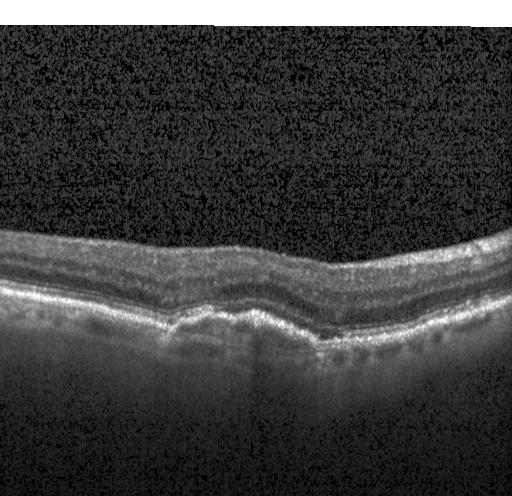
Impression: CNV.